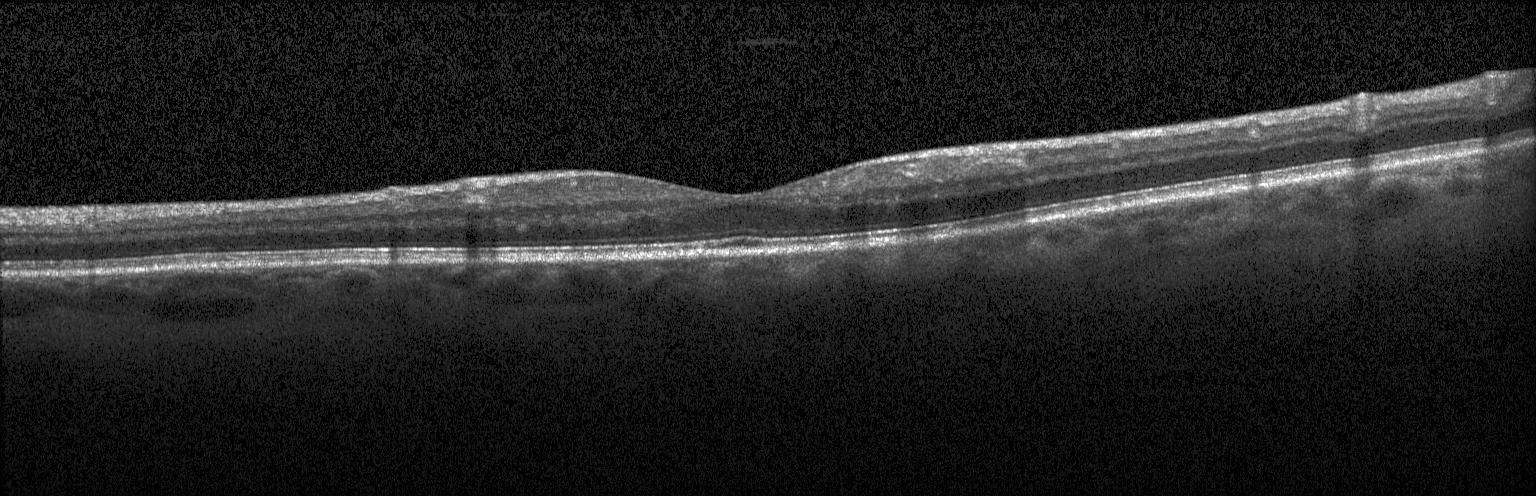
Spectral-domain OCT, retinal OCT cross-section, Heidelberg Spectralis OCT system
Finding: neither choroidal neovascularization, diabetic macular edema, nor drusen.